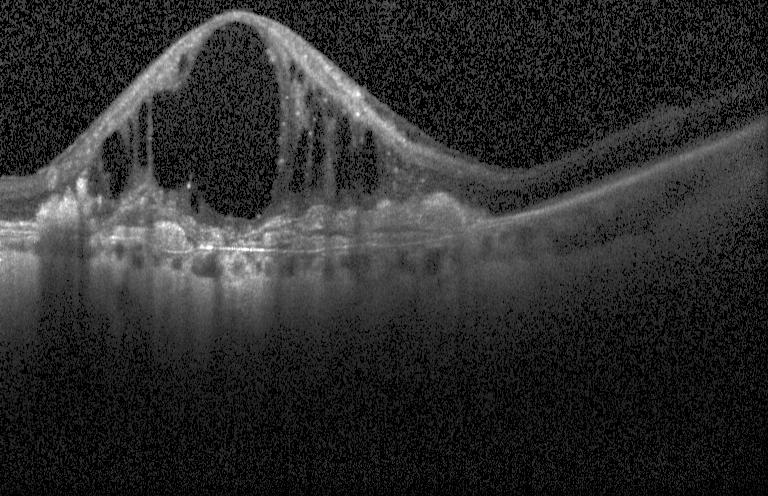 Fovea-centered. Spectral-domain optical coherence tomography. Optical coherence tomography B-scan — Diagnosis: choroidal neovascularization.